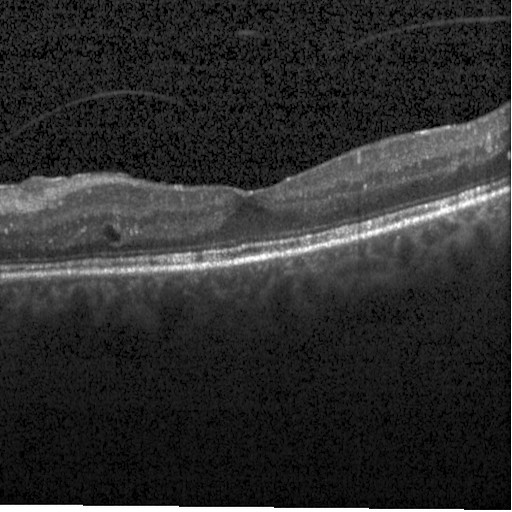 Spectral-domain optical coherence tomography · retinal OCT B-scan · macular scan
Dx: diabetic macular edema (DME).